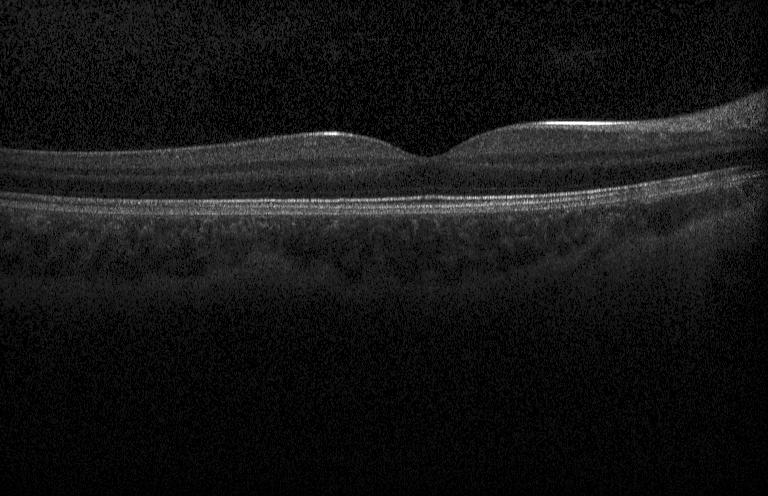 Assessment: no evidence of CNV, DME, or drusen.